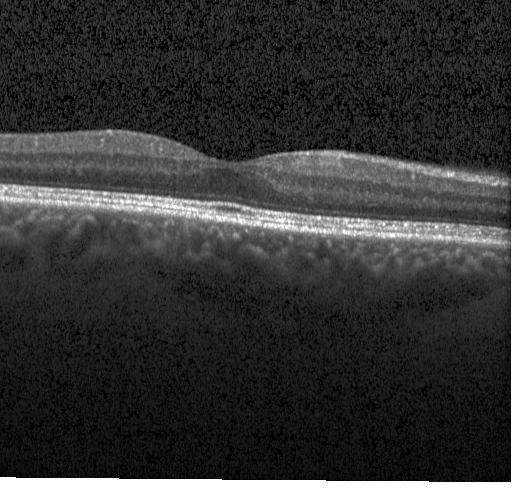

SD-OCT · optical coherence tomography scan · Heidelberg Spectralis OCT system · fovea-centered — No choroidal neovascularization, diabetic macular edema, or drusen.